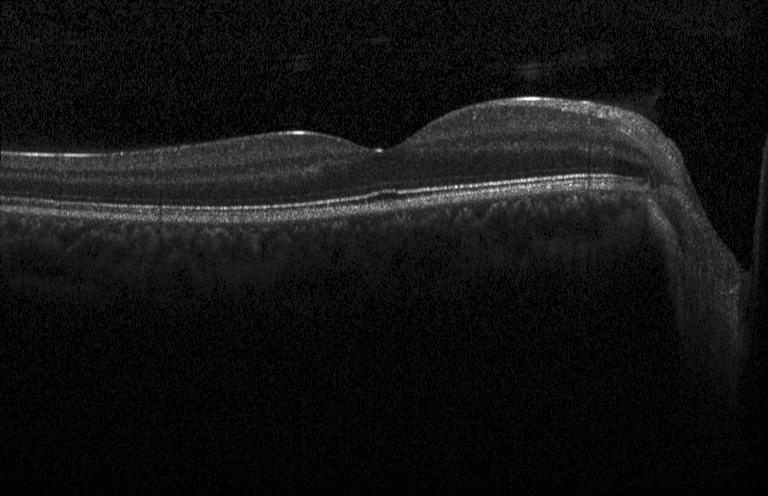
The scan shows neither choroidal neovascularization, diabetic macular edema, nor drusen.